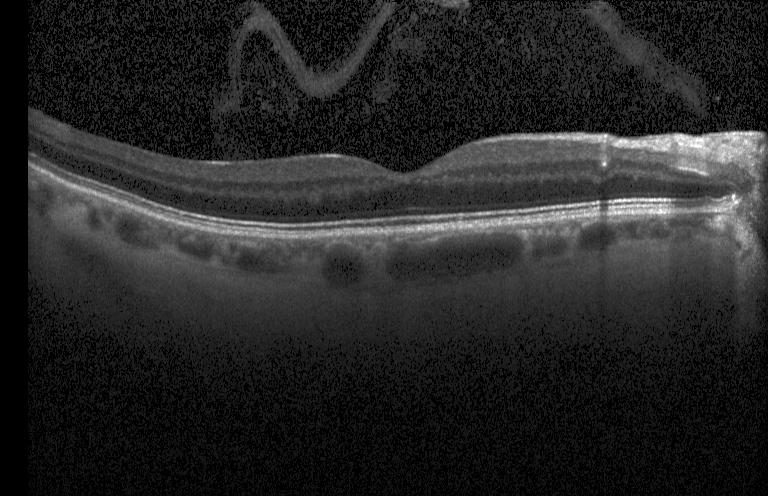 OCT B-scan, acquired on a Heidelberg Spectralis, through the macula, spectral-domain optical coherence tomography.
Diagnosis: neither choroidal neovascularization, diabetic macular edema, nor drusen.